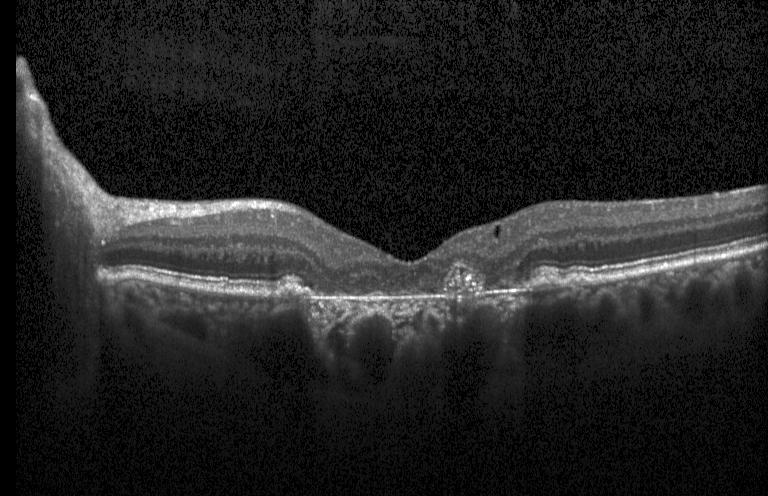 OCT line scan; centered on the fovea; spectral-domain OCT; instrument: Heidelberg Spectralis
Assessment: a choroidal neovascular membrane.